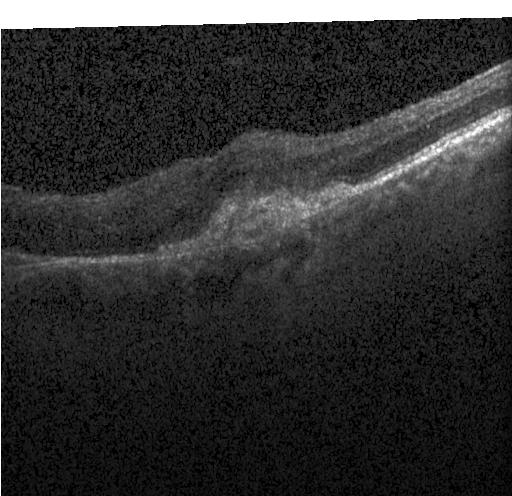
Diagnosis: CNV.